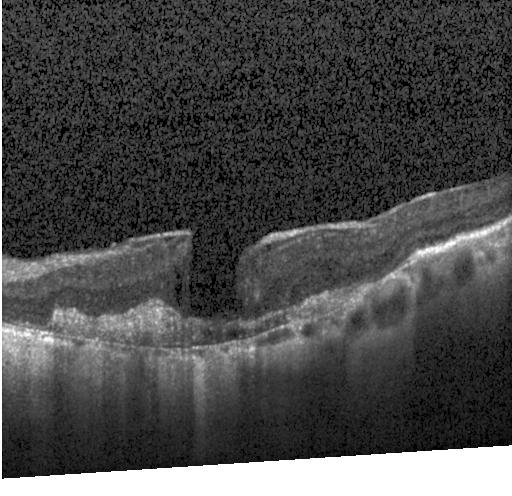 Retinal OCT B-scan. Macular scan. Heidelberg Spectralis OCT system. Spectral-domain OCT — Diagnosis: choroidal neovascularization.